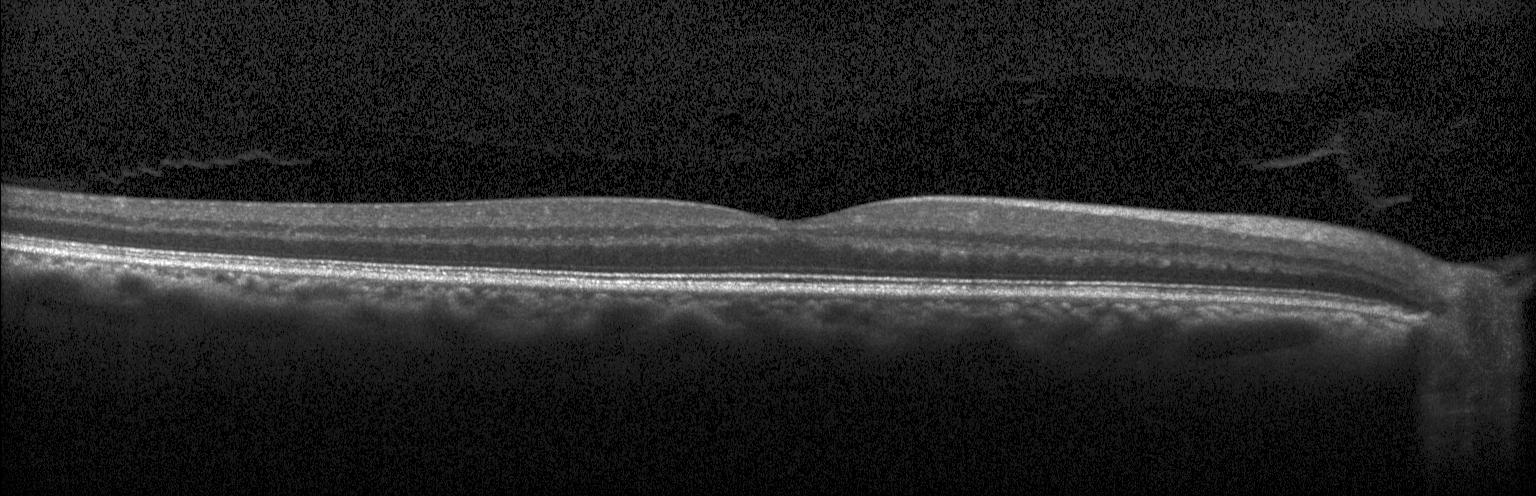 Centered on the fovea · retinal OCT cross-section · spectral-domain OCT · instrument: Heidelberg Spectralis.
Assessment: no CNV, no DME, and no drusen.